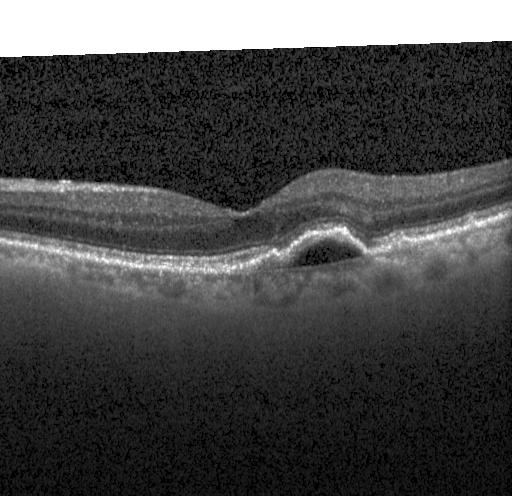 OCT B-scan.
Impression: a choroidal neovascular membrane.